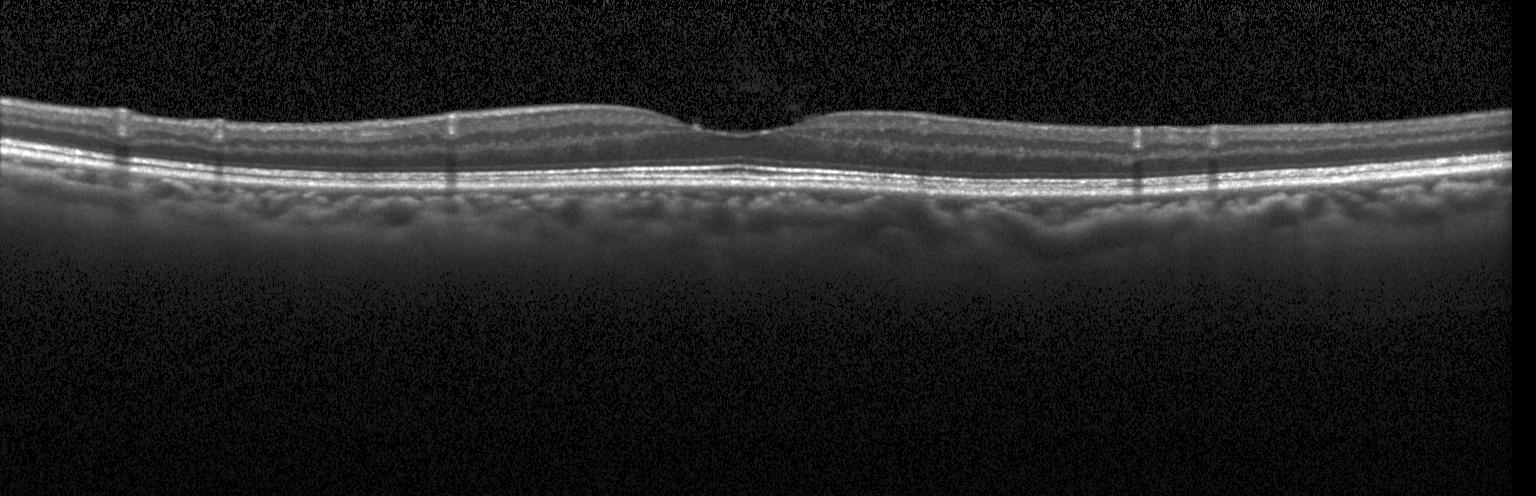

Neither CNV, DME, nor drusen.